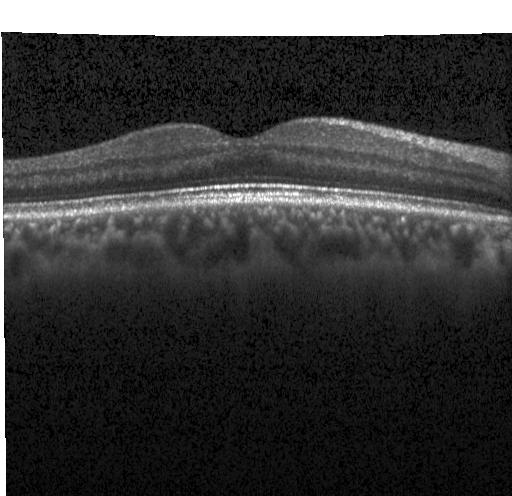
Diagnosis: no choroidal neovascularization, diabetic macular edema, or drusen.